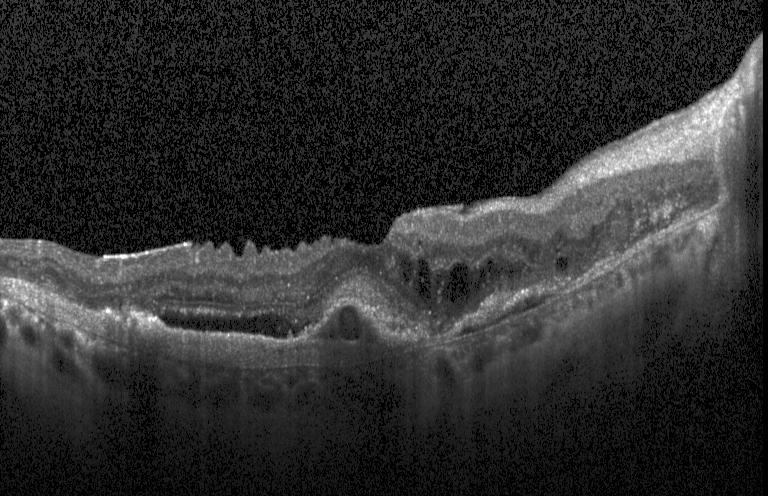
Diagnosis: a choroidal neovascular membrane.